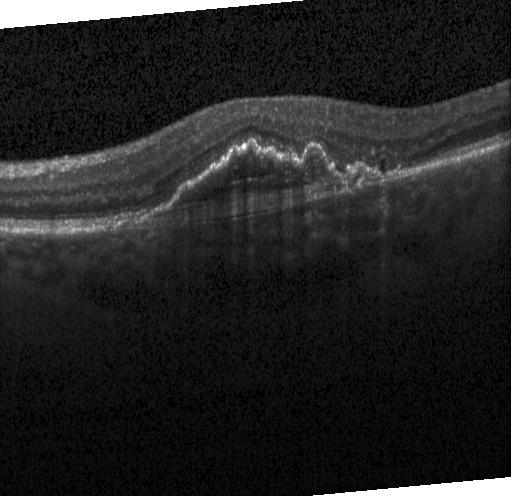

Finding: a choroidal neovascular membrane.